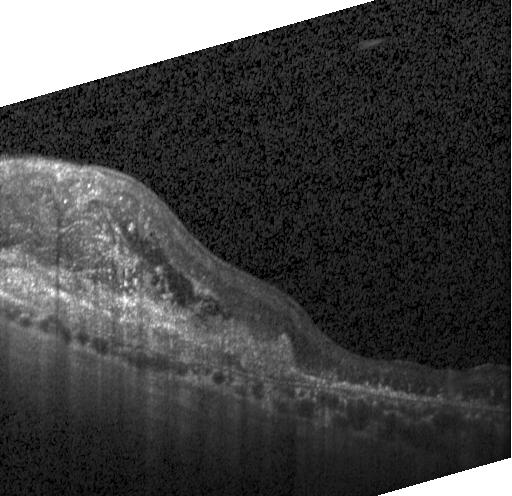

OCT finding: choroidal neovascularization.